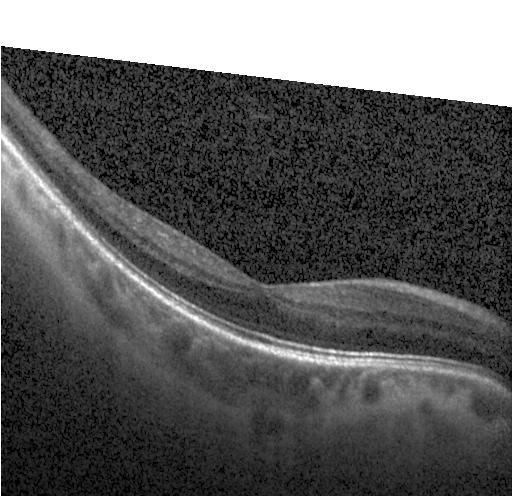 Impression: no choroidal neovascularization, diabetic macular edema, or drusen.